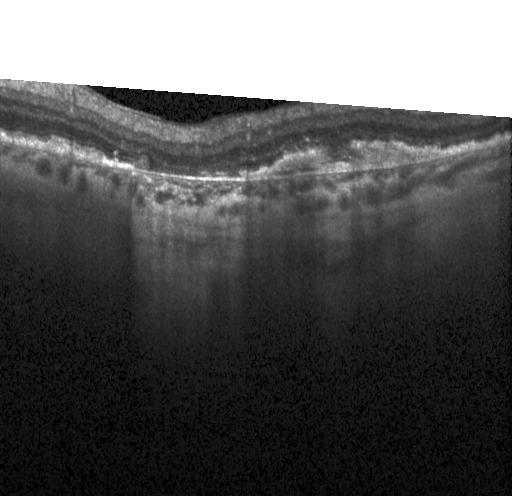
Through the macula · OCT line scan · acquired on a Heidelberg Spectralis · spectral-domain optical coherence tomography. This B-scan demonstrates CNV.